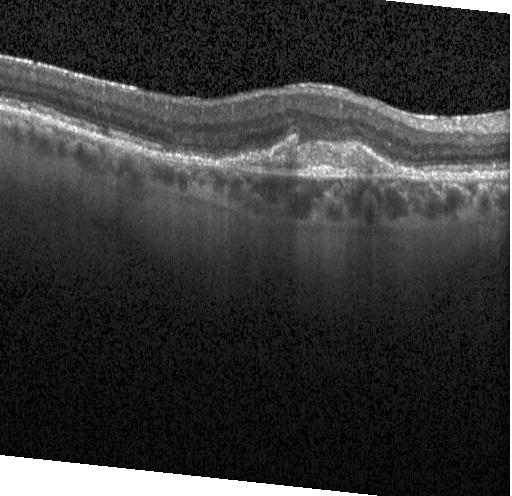 Spectral-domain OCT · optical coherence tomography scan · Heidelberg Spectralis · through the macula.
OCT finding: choroidal neovascularization.